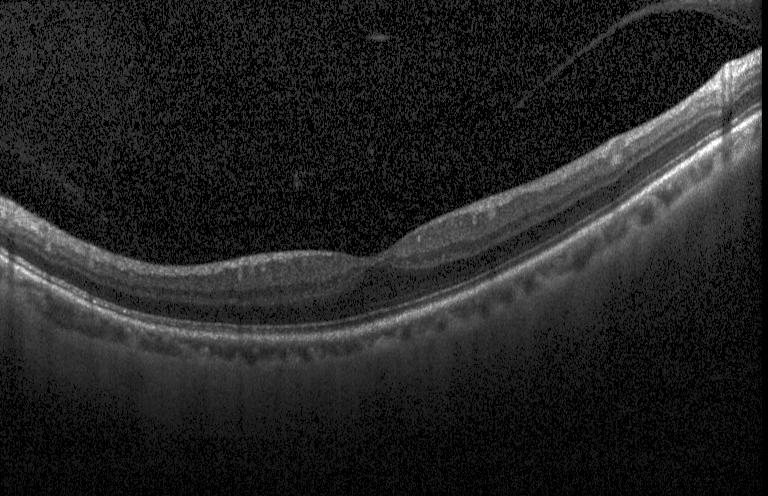

Retinal OCT cross-section showing no evidence of choroidal neovascularization, diabetic macular edema, or drusen.